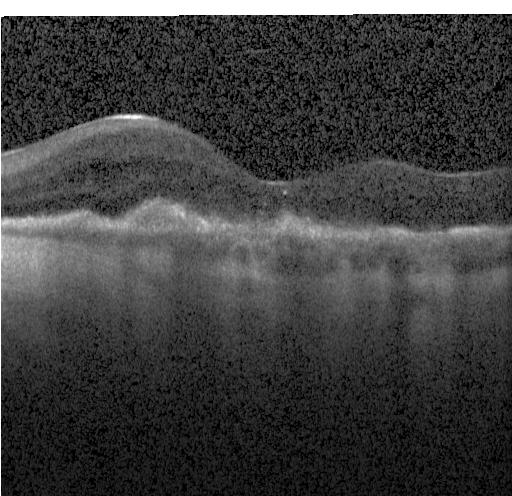 Macular OCT: CNV.